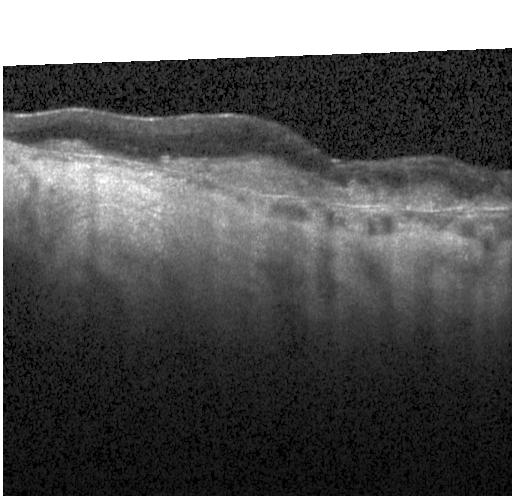 Diagnosis: choroidal neovascularization.